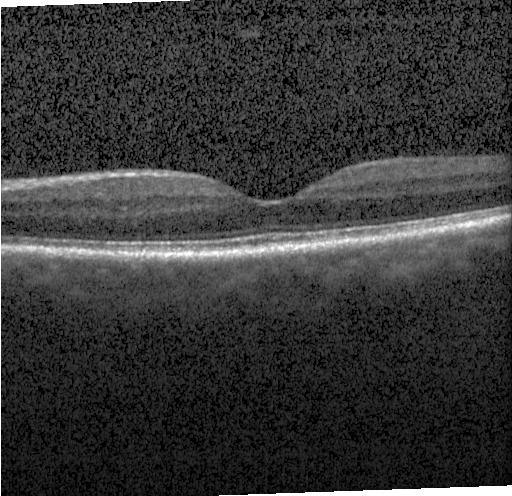
Diagnosis: no choroidal neovascularization, diabetic macular edema, or drusen.